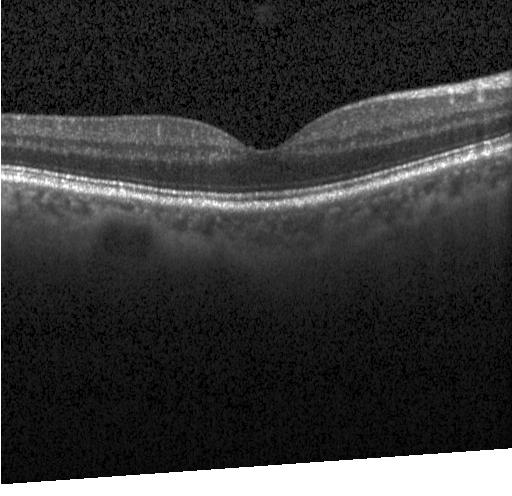 No CNV, DME, or drusen.